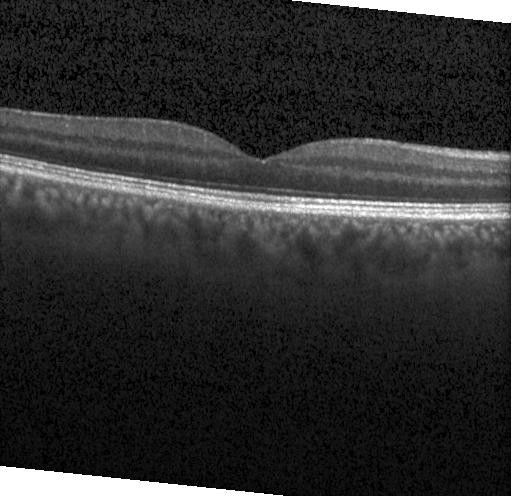 Heidelberg Spectralis OCT system, spectral-domain OCT, retinal OCT B-scan, macular scan.
This B-scan demonstrates no choroidal neovascularization, diabetic macular edema, or drusen.